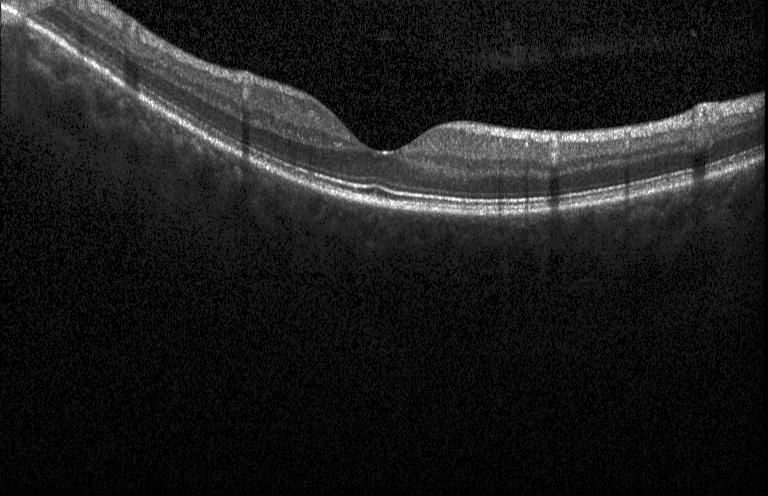
Retinal OCT cross-section. SD-OCT. Instrument: Heidelberg Spectralis
Diagnosis: neither choroidal neovascularization, diabetic macular edema, nor drusen.